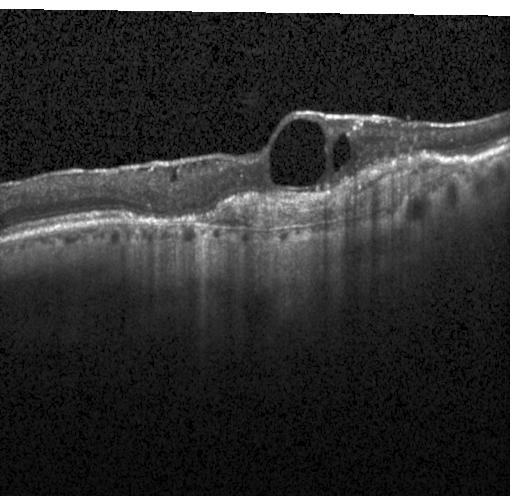

Optical coherence tomography B-scan, through the macula, Heidelberg Spectralis, SD-OCT. Finding: choroidal neovascularization (CNV).